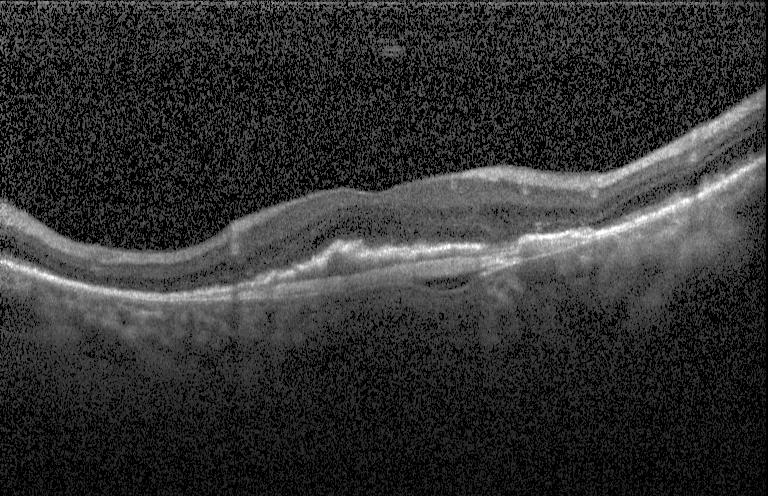

A choroidal neovascular membrane.